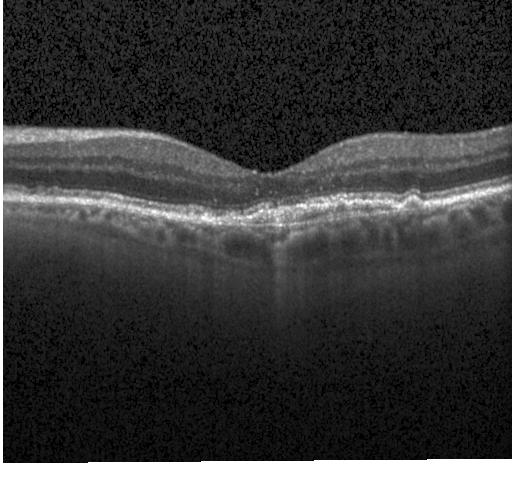

Spectral-domain OCT. OCT B-scan. Fovea-centered. This B-scan demonstrates choroidal neovascularization.